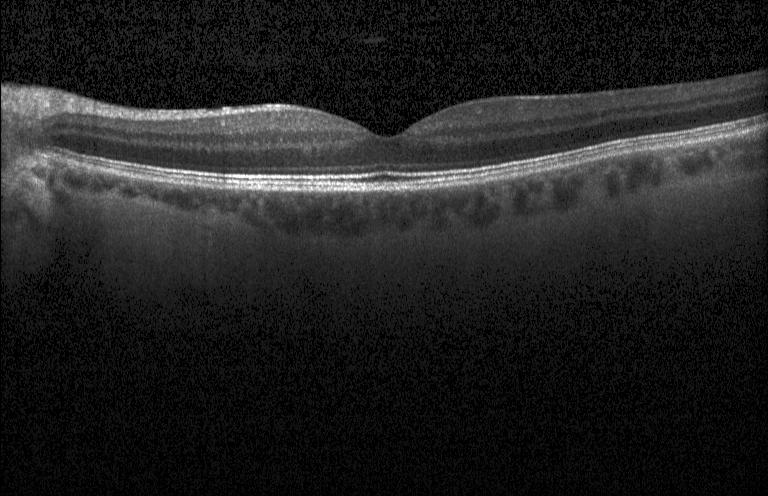

Dx: no evidence of CNV, DME, or drusen.